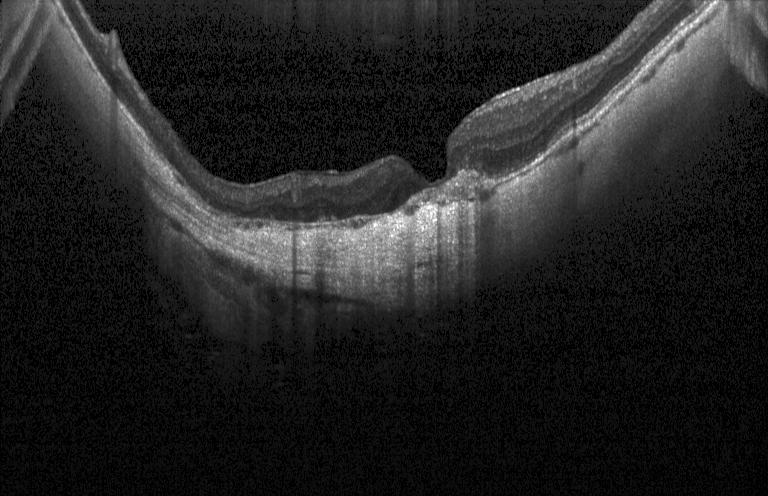 Acquired on a Heidelberg Spectralis. Retinal OCT B-scan
A choroidal neovascular membrane.